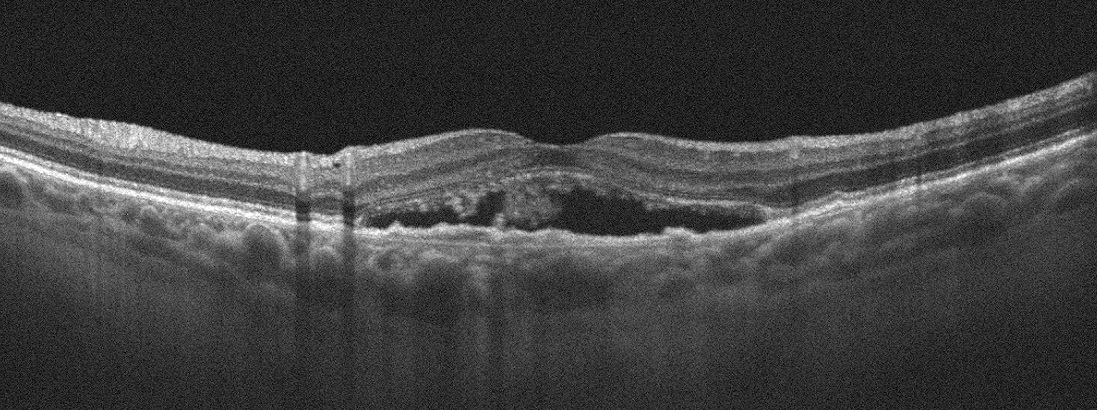 Finding: AMD.